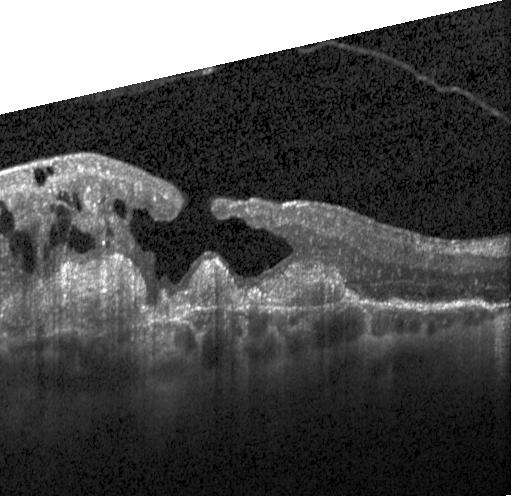 Instrument: Heidelberg Spectralis · optical coherence tomography B-scan · fovea-centered. Macular OCT: choroidal neovascularization.